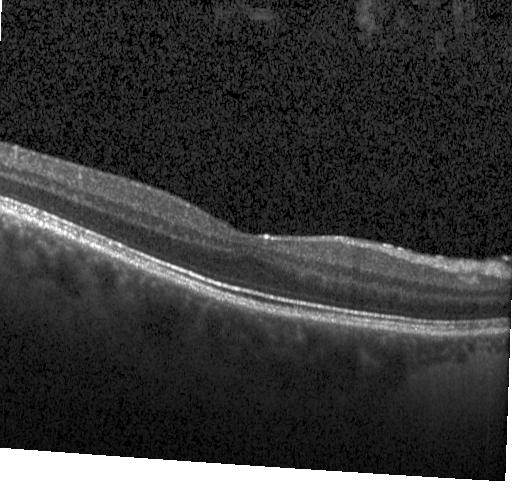 OCT line scan. Finding: neither choroidal neovascularization, diabetic macular edema, nor drusen.